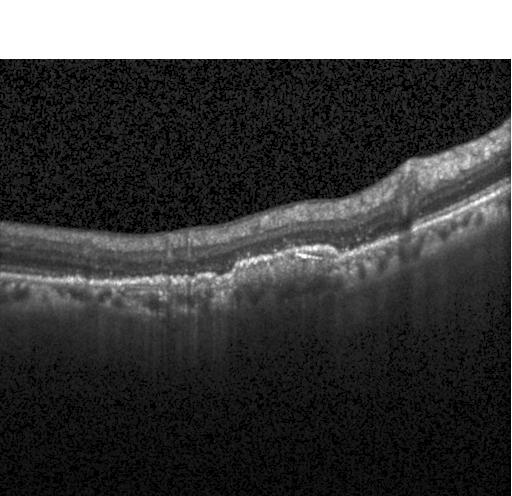
OCT scan showing a choroidal neovascular membrane.